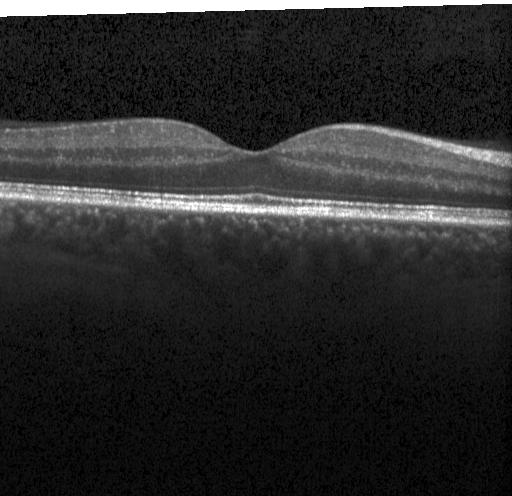 Retinal OCT cross-section, instrument: Heidelberg Spectralis.
The scan shows neither CNV, DME, nor drusen.